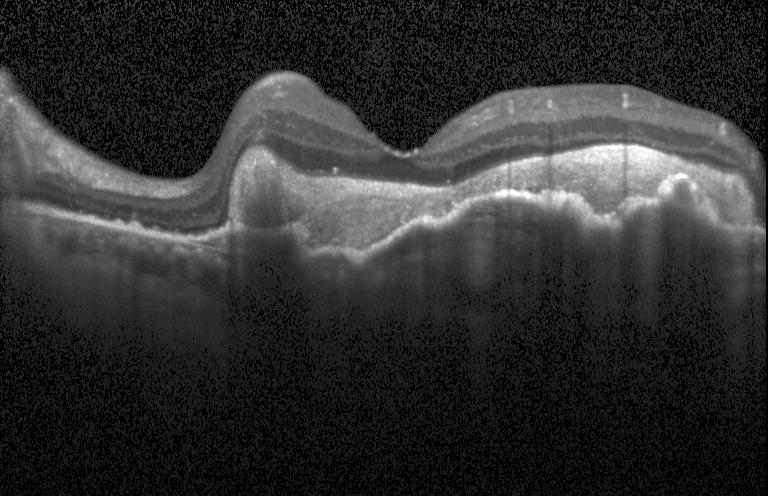

A choroidal neovascular membrane.